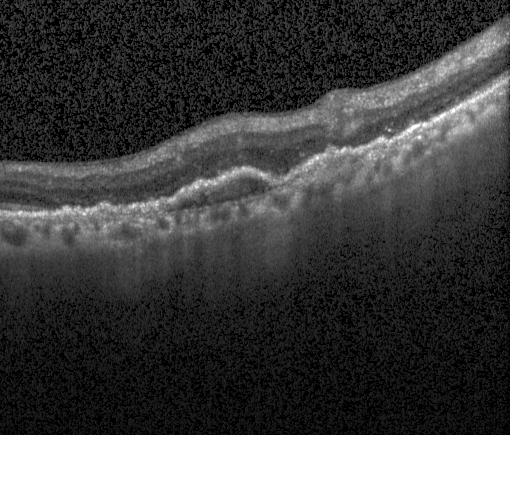 Retinal OCT B-scan. Heidelberg Spectralis OCT system. Fovea-centered. Spectral-domain optical coherence tomography
Impression: a choroidal neovascular membrane.